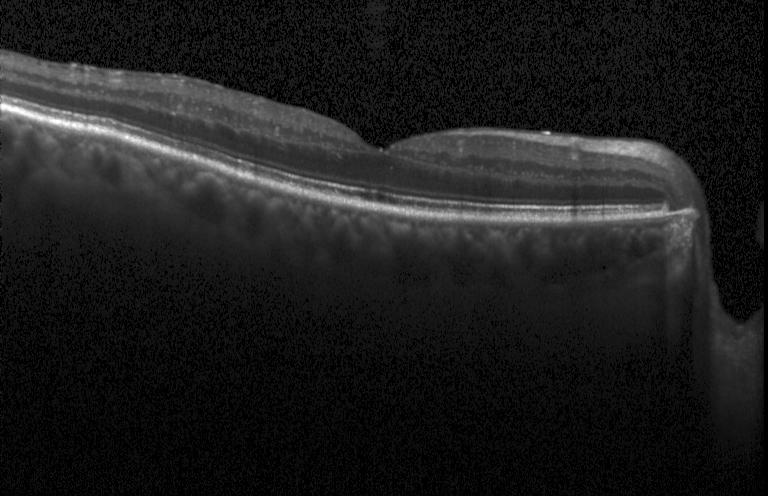

Macular OCT: no choroidal neovascularization, no diabetic macular edema, and no drusen.